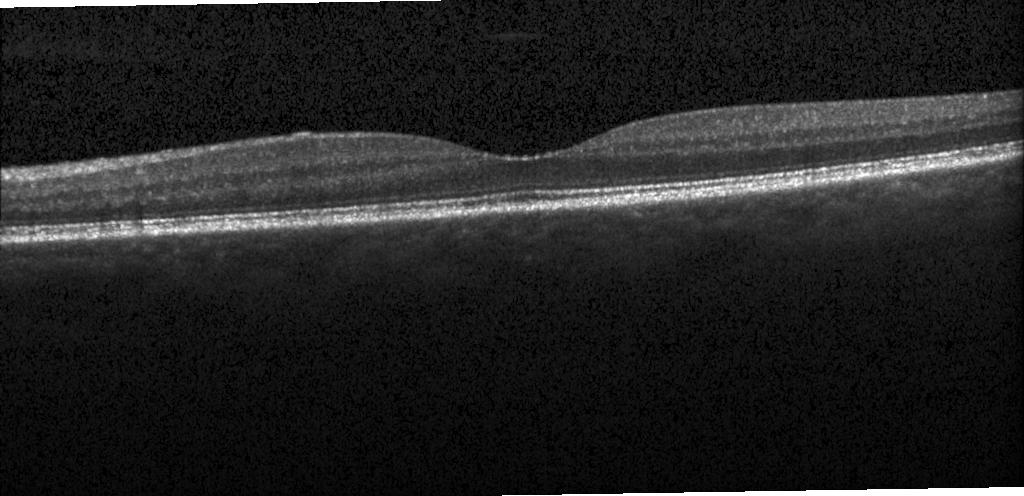
Macular OCT: no choroidal neovascularization, no diabetic macular edema, and no drusen.